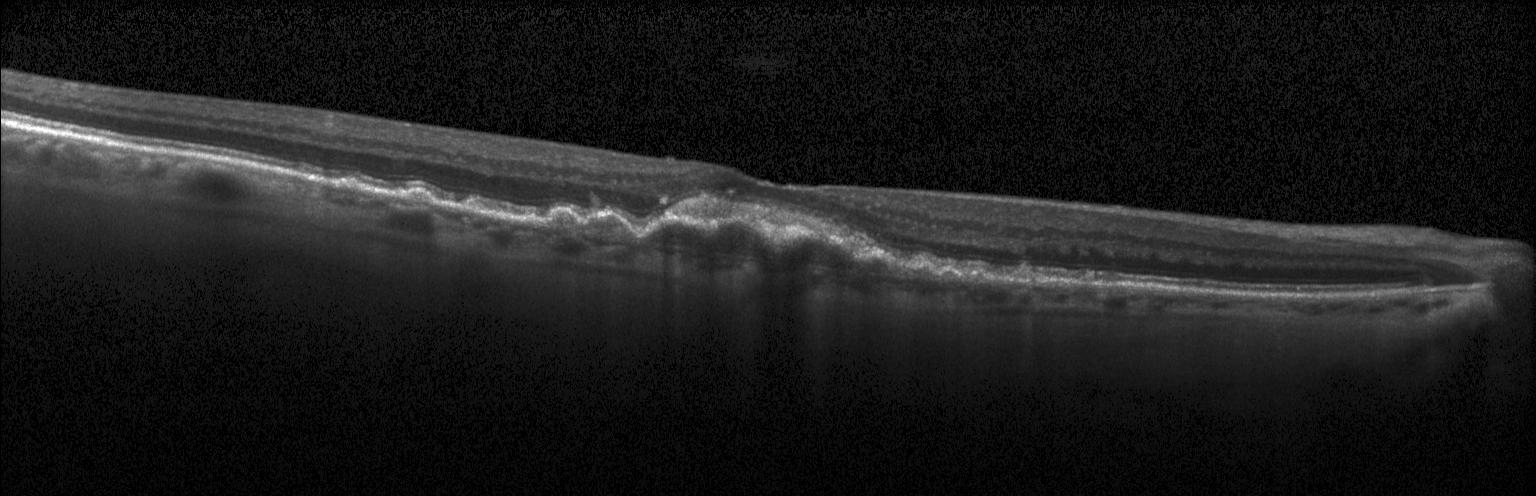 Heidelberg Spectralis OCT system. Macular scan. OCT line scan. Impression: CNV.